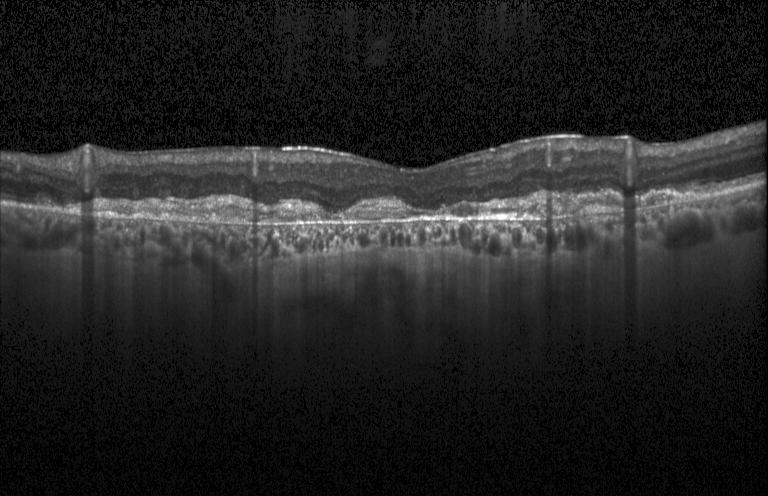 Finding: a choroidal neovascular membrane.